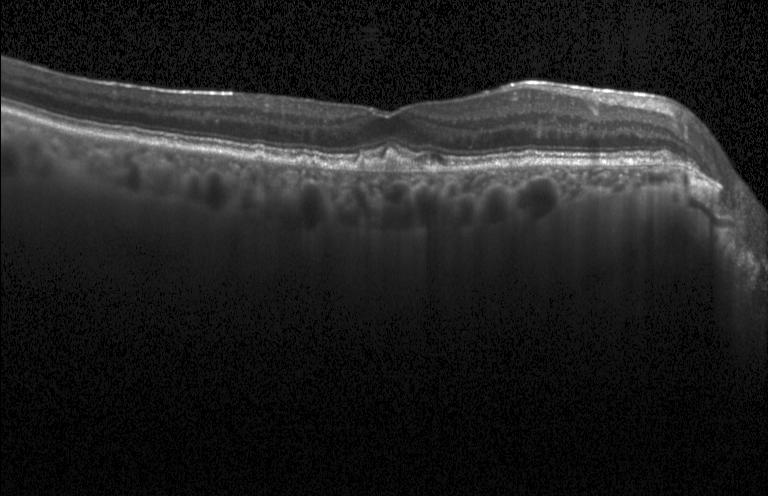
Impression: drusen.